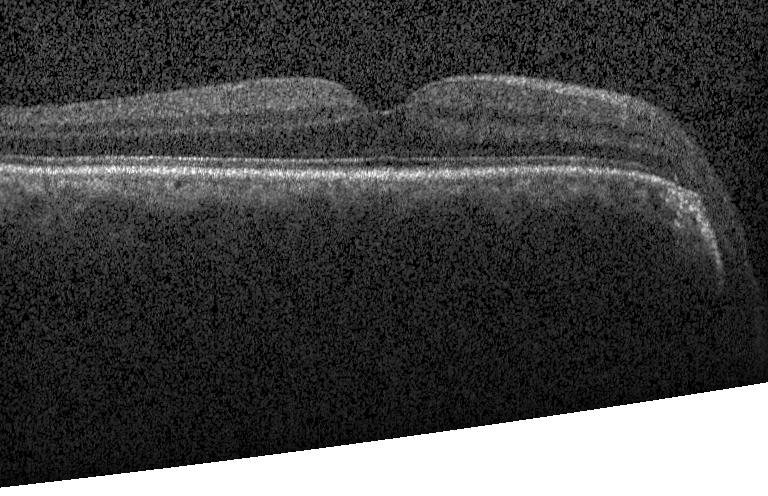 Spectral-domain OCT B-scan: neither choroidal neovascularization, diabetic macular edema, nor drusen.